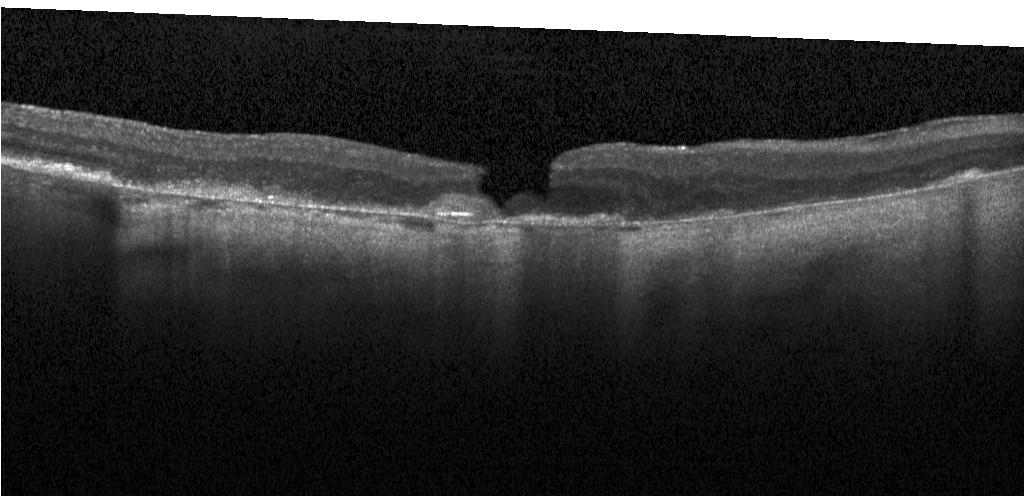
Spectral-domain optical coherence tomography. Heidelberg Spectralis. Optical coherence tomography scan. Macular scan
Diagnosis: CNV.